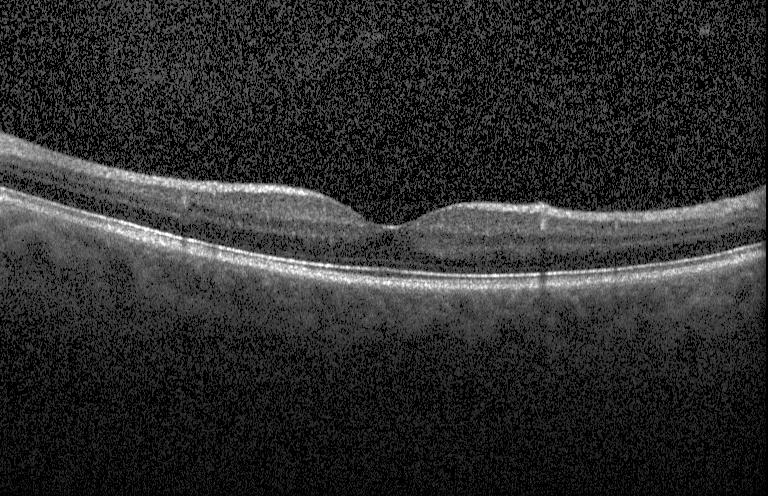

Acquired on a Heidelberg Spectralis; optical coherence tomography B-scan; spectral-domain optical coherence tomography; macular scan
Diagnosis: no choroidal neovascularization, no diabetic macular edema, and no drusen.